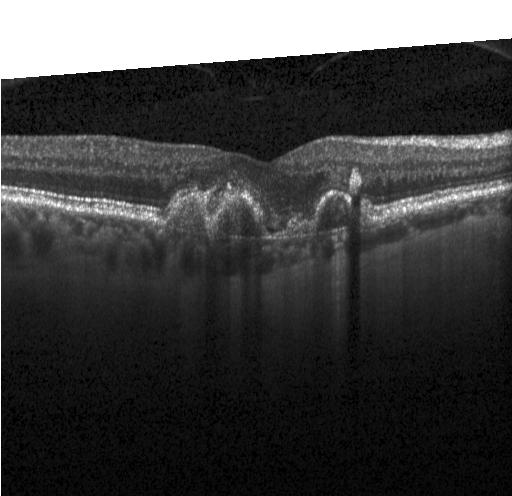 Retinal OCT B-scan. Assessment: choroidal neovascularization.